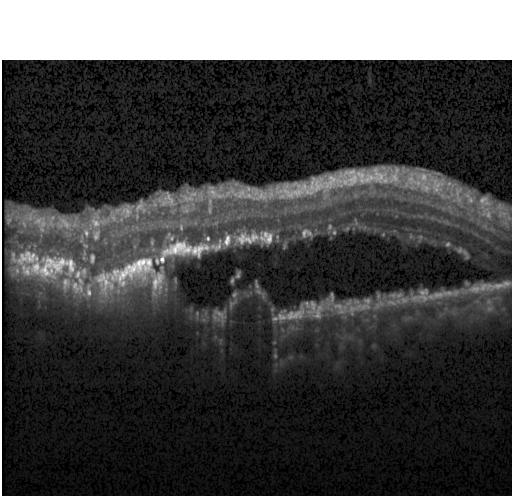
Macular OCT demonstrating a choroidal neovascular membrane.